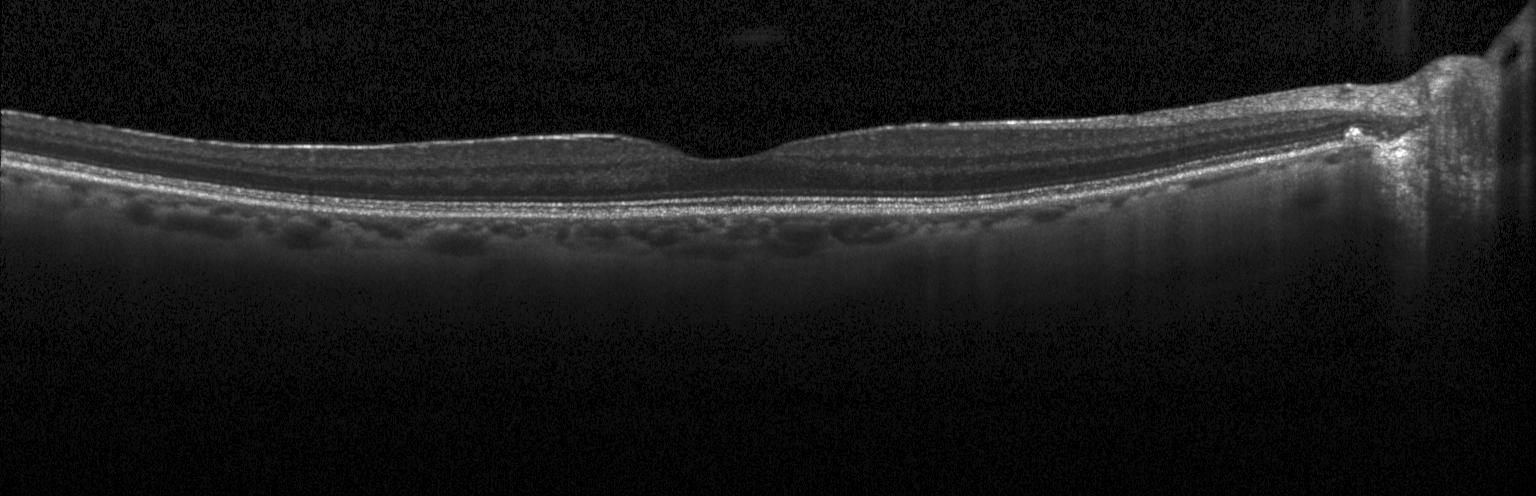
Spectral-domain OCT B-scan: no evidence of choroidal neovascularization, diabetic macular edema, or drusen.